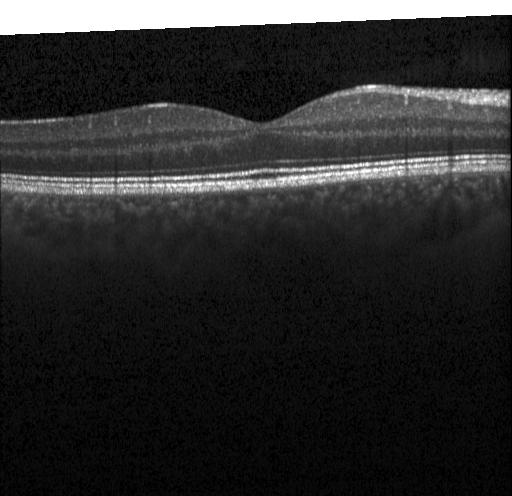
Centered on the fovea · OCT line scan. Impression: no CNV, DME, or drusen.